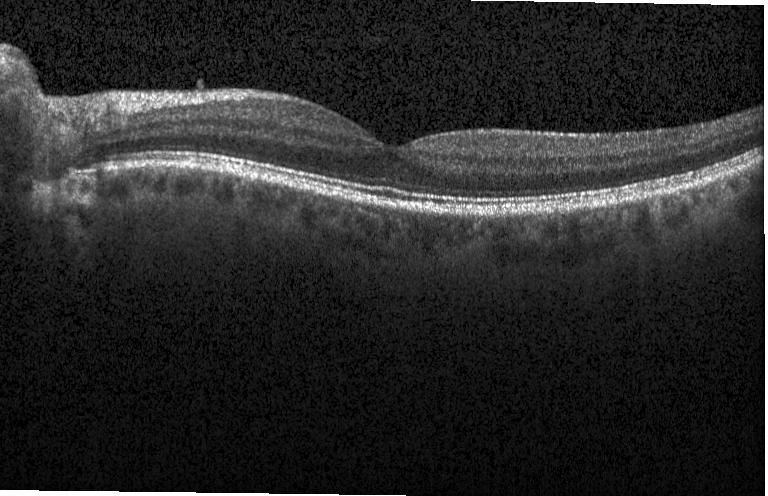

Through the macula · optical coherence tomography B-scan · Heidelberg Spectralis OCT system
This B-scan demonstrates no CNV, no DME, and no drusen.